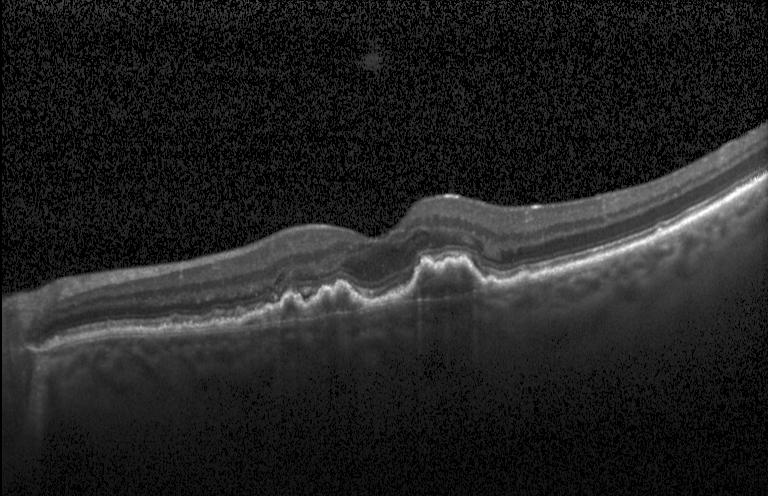

Spectral-domain OCT B-scan: choroidal neovascularization (CNV).